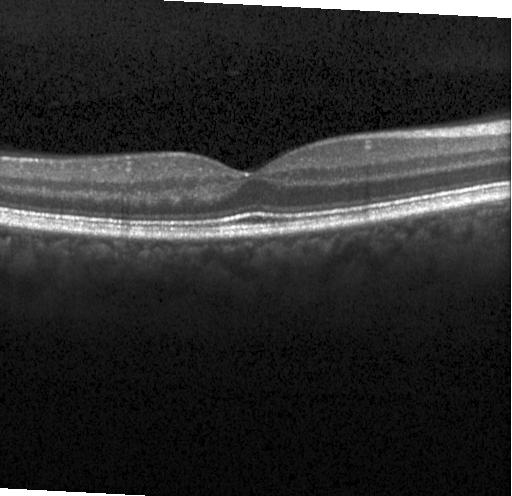

Optical coherence tomography scan · through the macula
Macular OCT: no choroidal neovascularization, no diabetic macular edema, and no drusen.